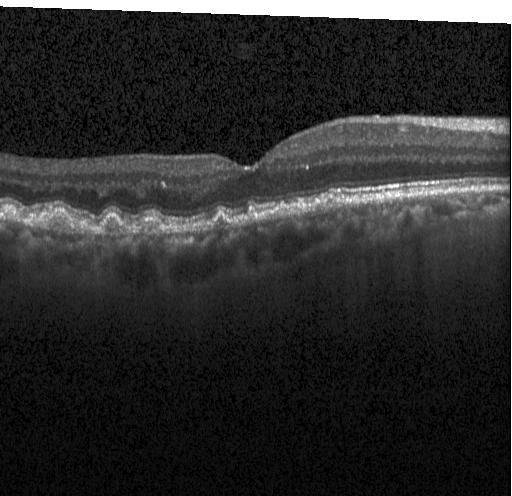

OCT line scan. Finding: sub-RPE drusenoid deposits.